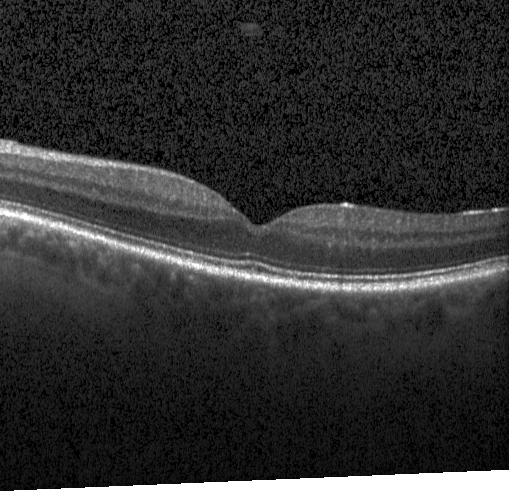
OCT line scan. Heidelberg Spectralis. Finding: no choroidal neovascularization, no diabetic macular edema, and no drusen.